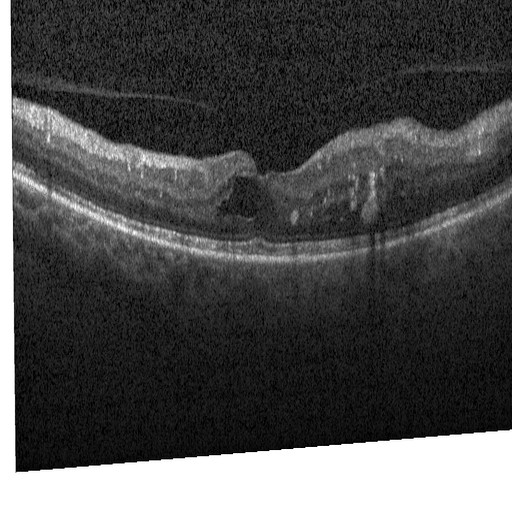

Assessment: diabetic macular edema.